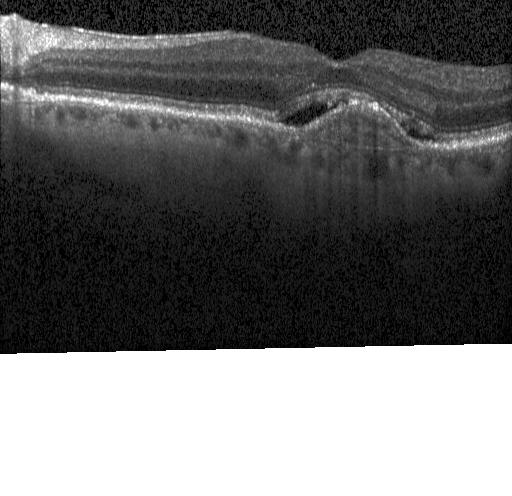
OCT line scan
Dx: CNV.